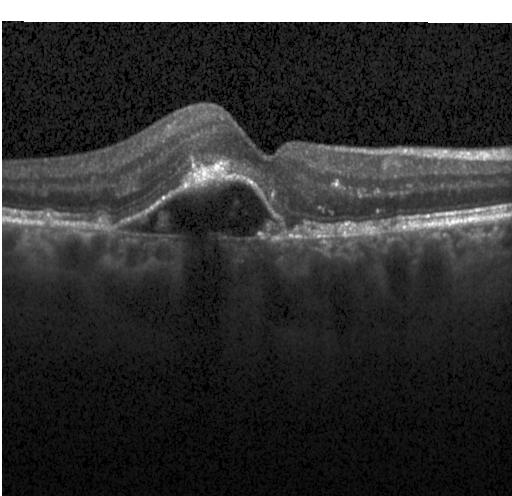 Spectral-domain optical coherence tomography, retinal OCT cross-section, centered on the fovea, instrument: Heidelberg Spectralis.
Diagnosis: a choroidal neovascular membrane.